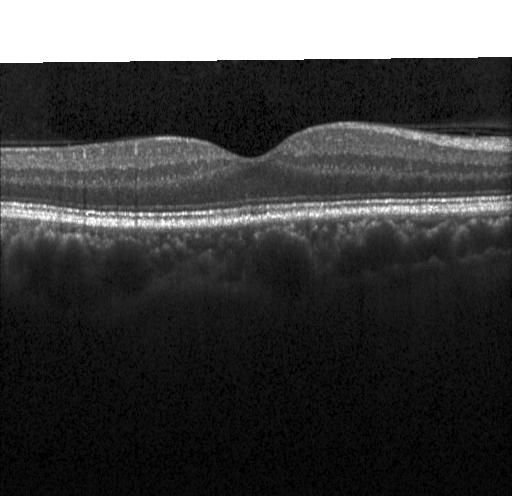
Assessment: no evidence of choroidal neovascularization, diabetic macular edema, or drusen.